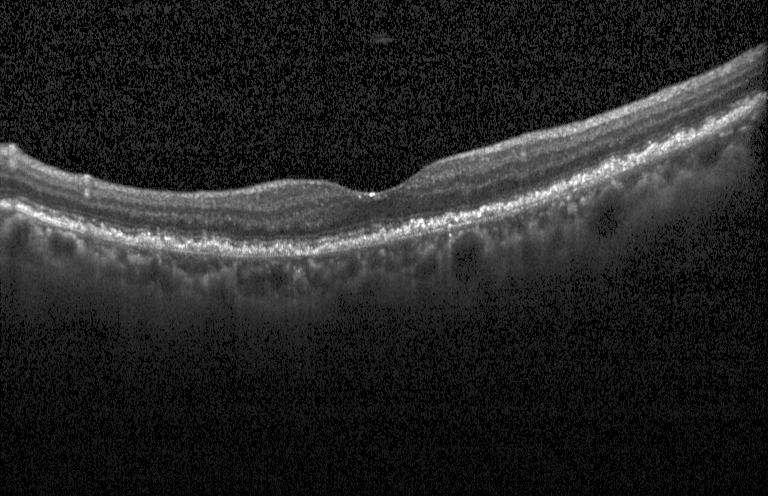 OCT scan showing drusen.